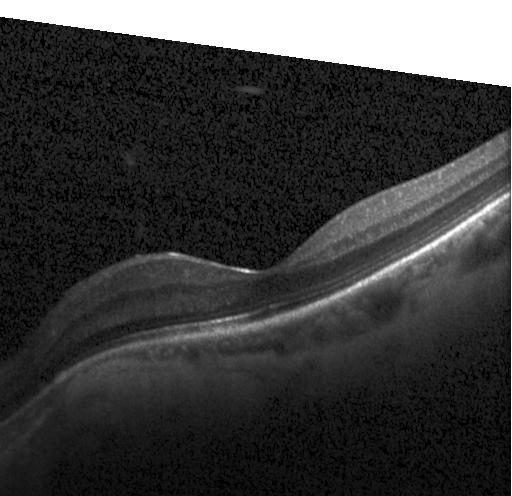
OCT B-scan · instrument: Heidelberg Spectralis. Diagnosis: neither choroidal neovascularization, diabetic macular edema, nor drusen.